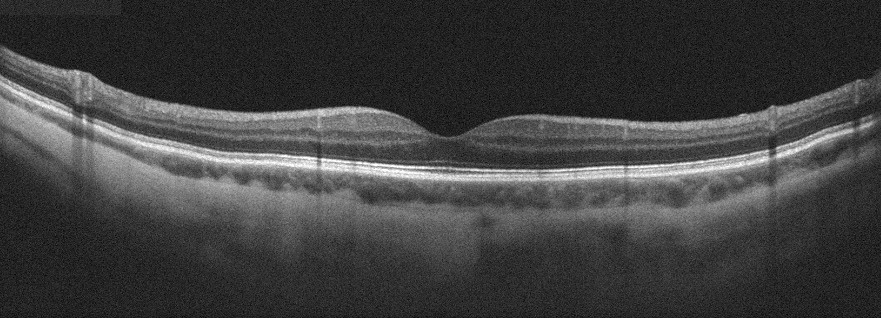 Optovue Avanti RTVue XR; macular scan; retinal OCT cross-section
Impression: no evidence of AMD, DME, ERM, RAO, RVO, or VID.